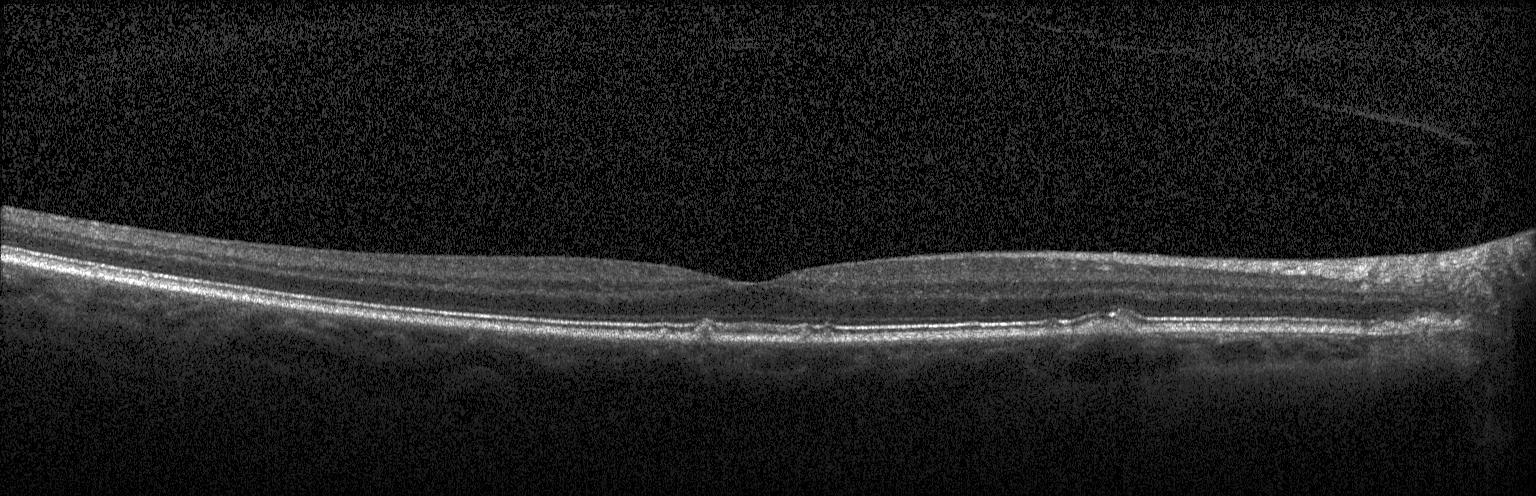

Impression: drusen.